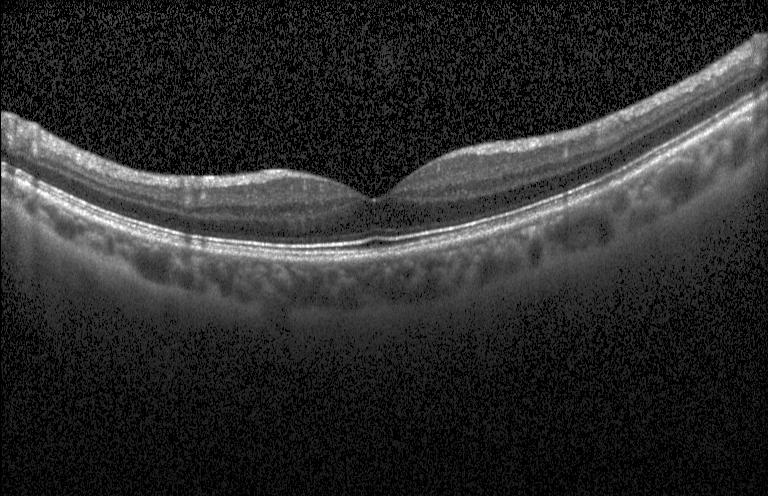

Spectral-domain OCT. Heidelberg Spectralis OCT system. Optical coherence tomography B-scan — Impression: no evidence of CNV, DME, or drusen.